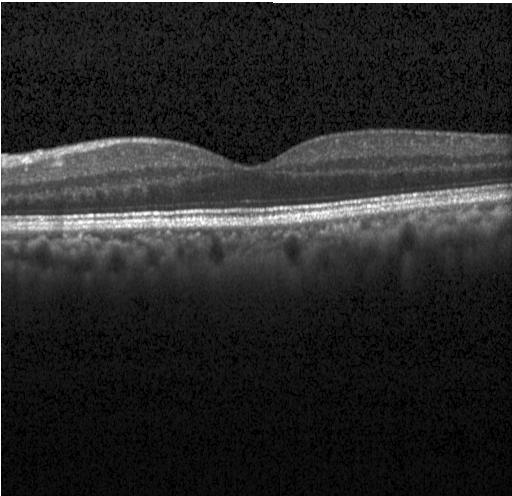 Retinal OCT cross-section.
Diagnosis: neither CNV, DME, nor drusen.